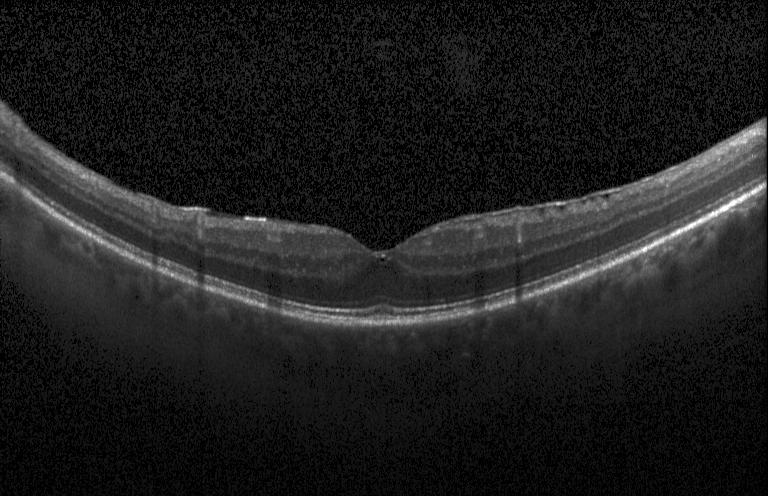 Spectral-domain OCT, macular scan, optical coherence tomography B-scan. Diagnosis: no choroidal neovascularization, diabetic macular edema, or drusen.